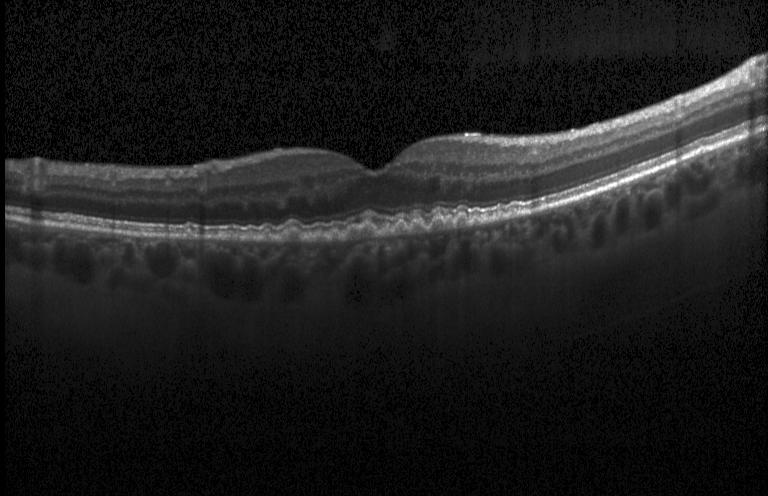
Fovea-centered · retinal OCT B-scan
OCT finding: sub-RPE drusenoid deposits.